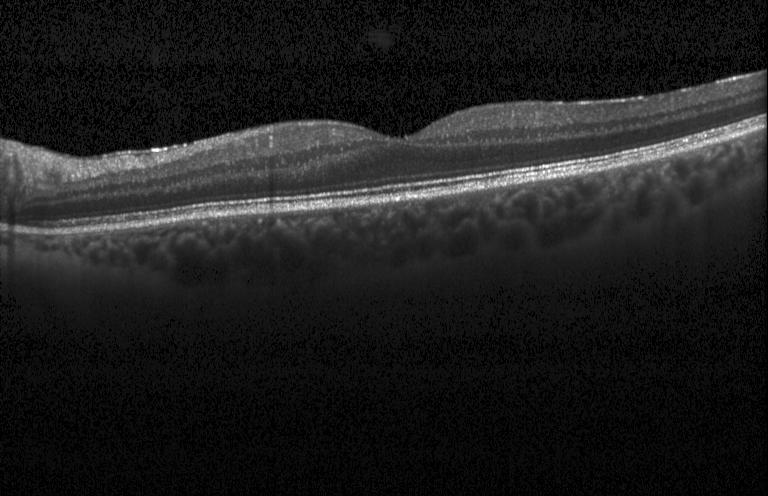
OCT B-scan. SD-OCT.
Finding: no choroidal neovascularization, no diabetic macular edema, and no drusen.